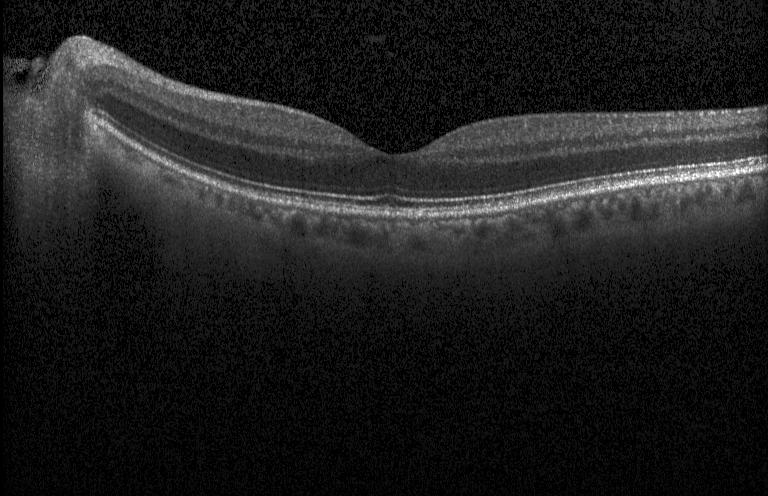
Finding: no CNV, DME, or drusen.